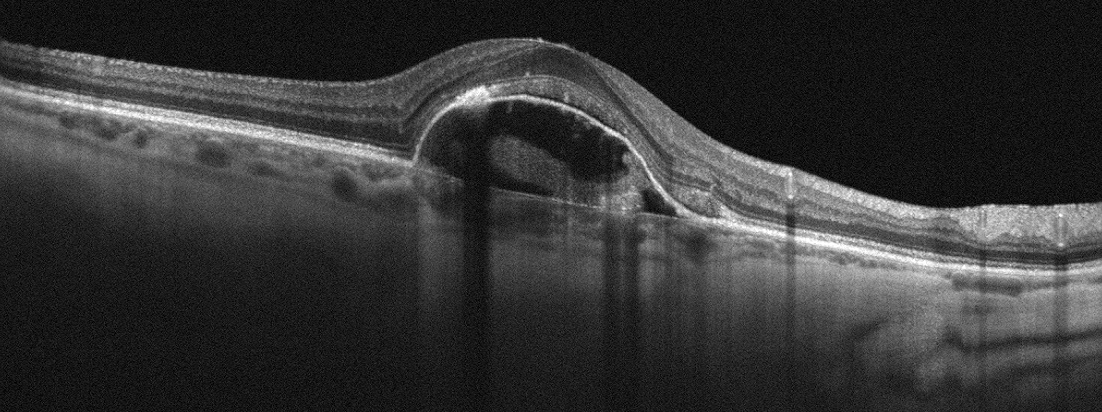

This B-scan demonstrates age-related macular degeneration.